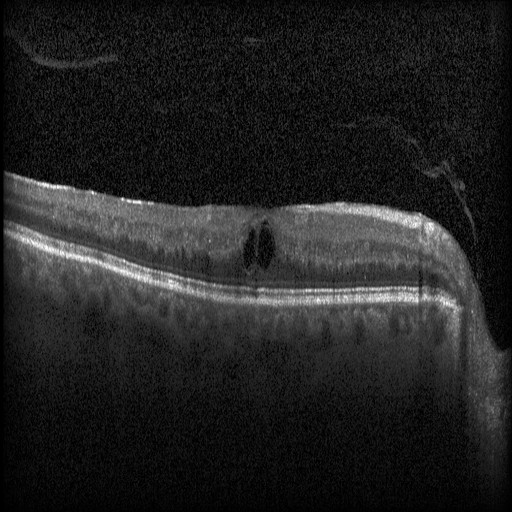

SD-OCT · retinal OCT B-scan · macular scan · Heidelberg Spectralis OCT system — Macular OCT: diabetic macular edema (DME).